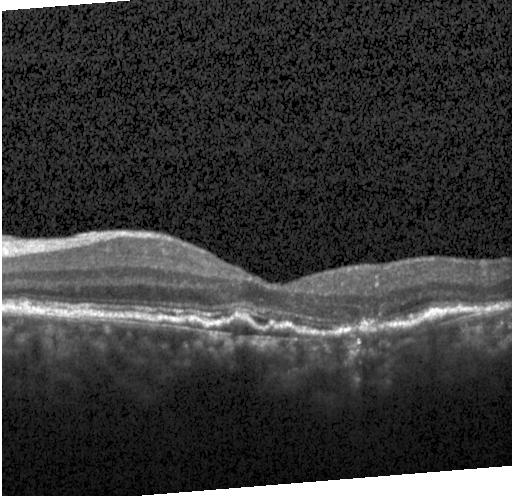
OCT line scan. SD-OCT. Through the macula. Heidelberg Spectralis OCT system
This B-scan demonstrates a choroidal neovascular membrane.